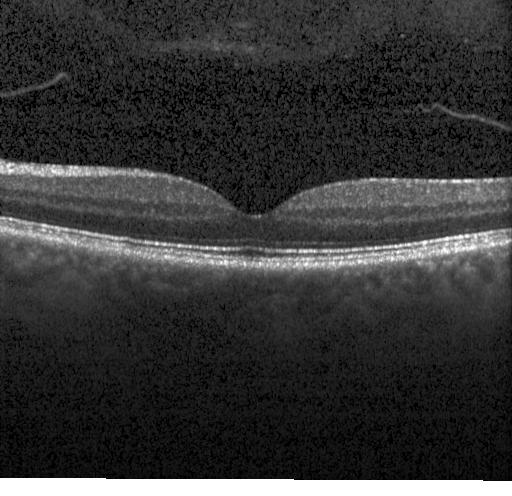

This B-scan demonstrates neither CNV, DME, nor drusen.